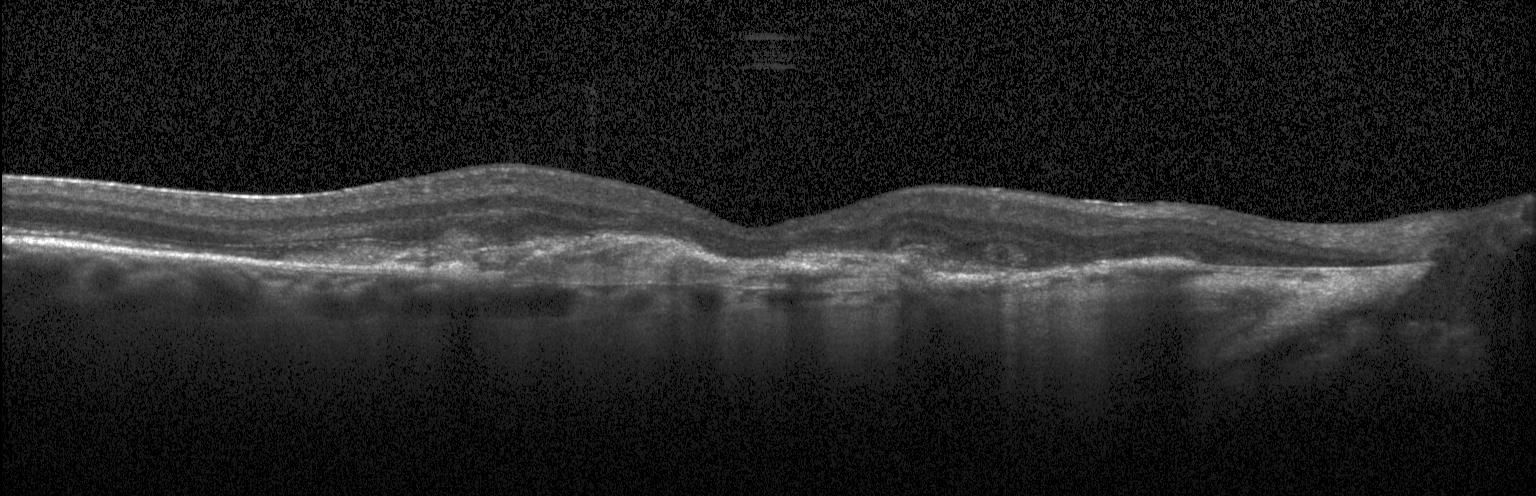 Diagnosis: a choroidal neovascular membrane.